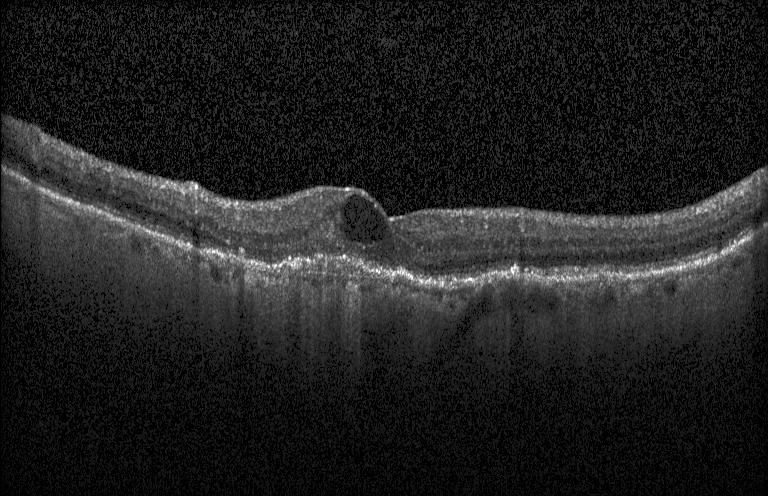 OCT line scan
The scan shows a choroidal neovascular membrane.